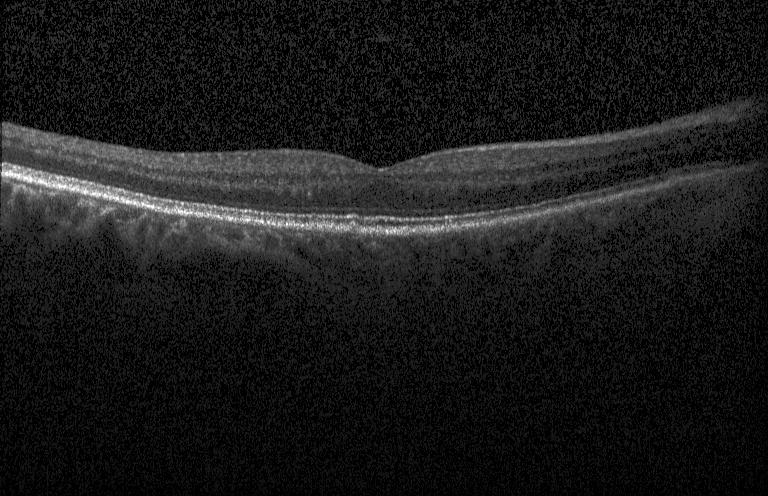 SD-OCT; optical coherence tomography scan.
Finding: no evidence of choroidal neovascularization, diabetic macular edema, or drusen.